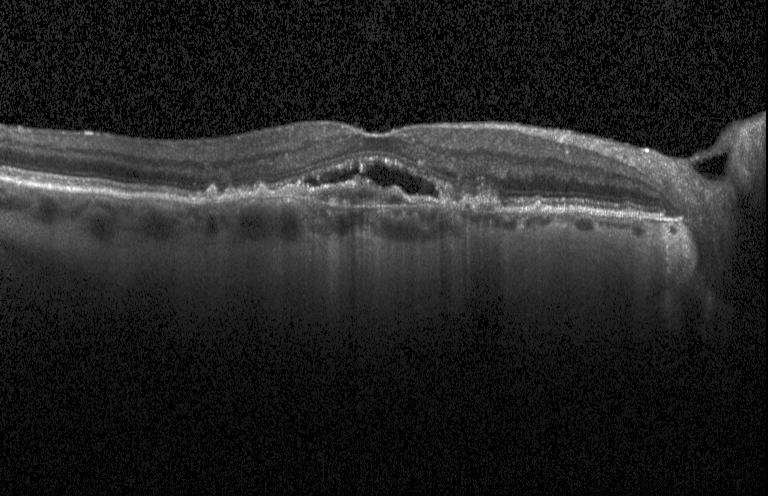 Macular OCT: choroidal neovascularization (CNV).